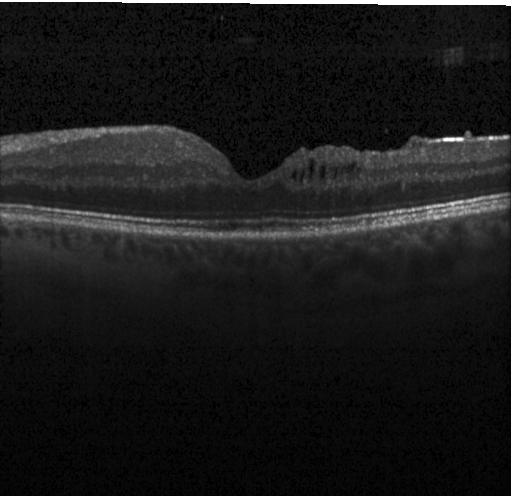 Instrument: Heidelberg Spectralis · OCT B-scan. DME.